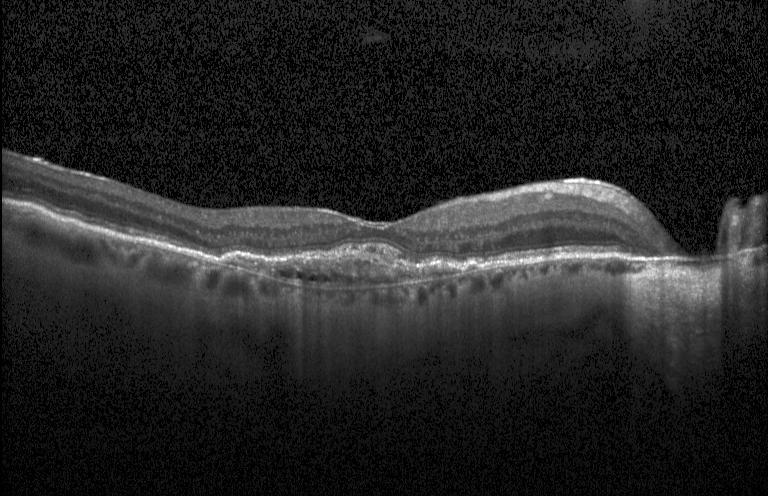
SD-OCT; acquired on a Heidelberg Spectralis; optical coherence tomography B-scan — Finding: CNV.